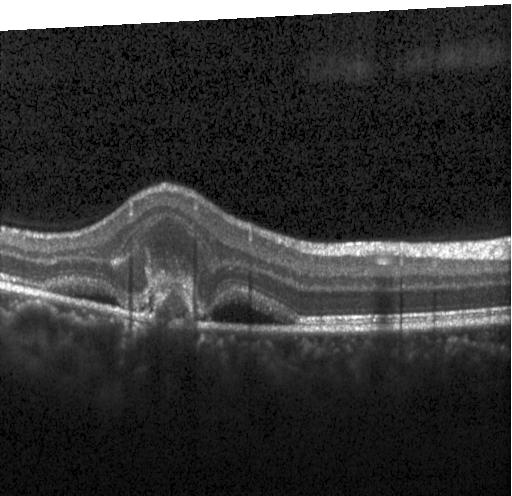 The scan shows choroidal neovascularization.